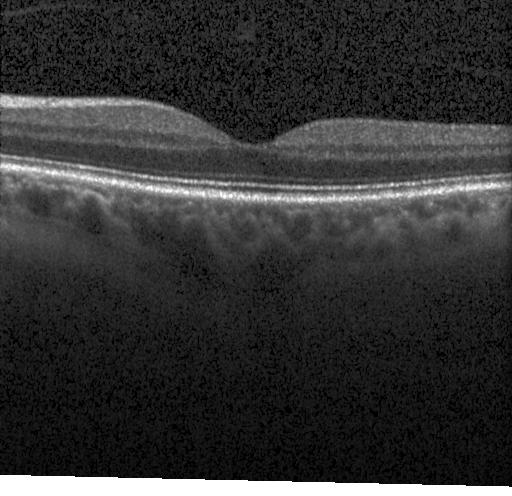 OCT scan showing no CNV, no DME, and no drusen.